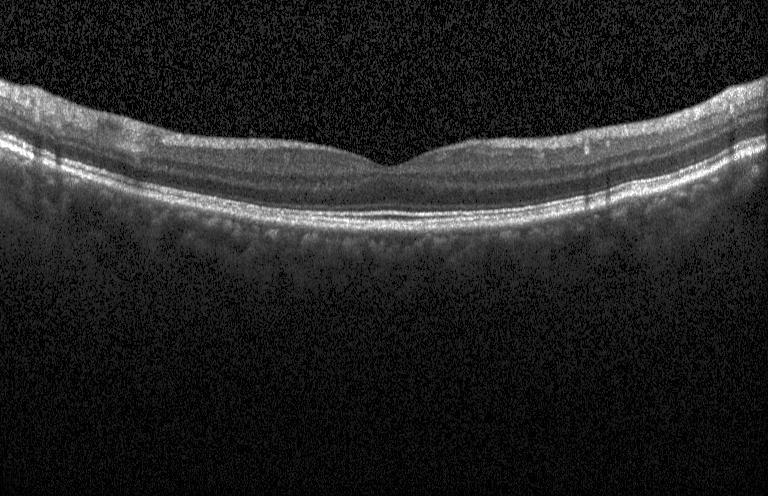 Optical coherence tomography B-scan
This B-scan demonstrates neither choroidal neovascularization, diabetic macular edema, nor drusen.